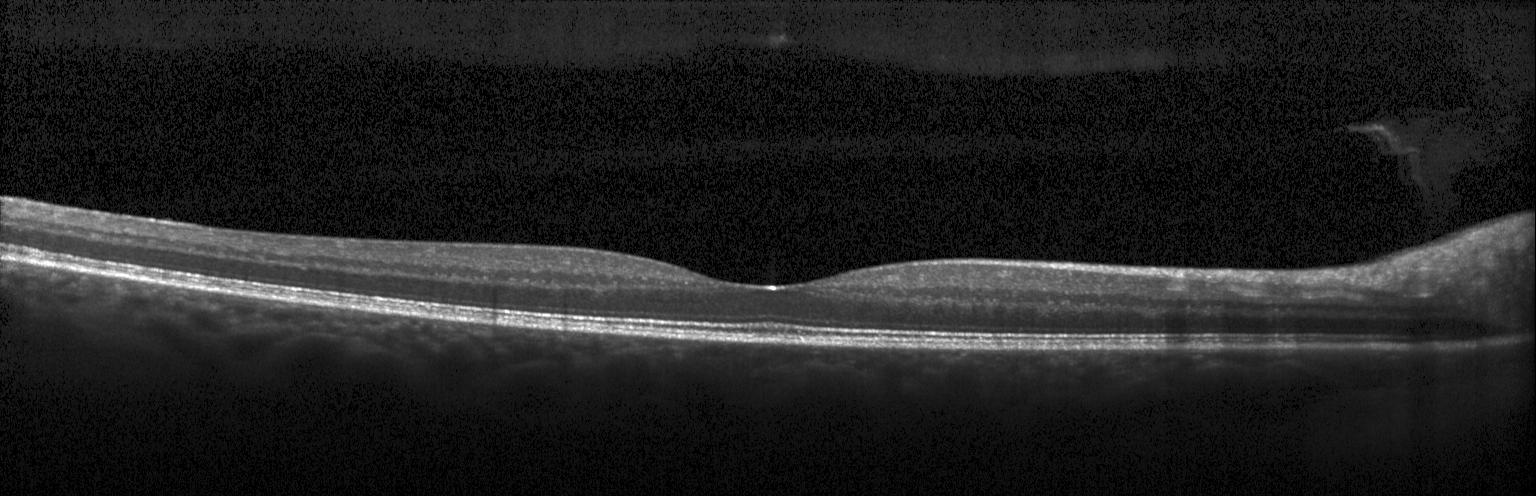
Macular OCT: neither CNV, DME, nor drusen.